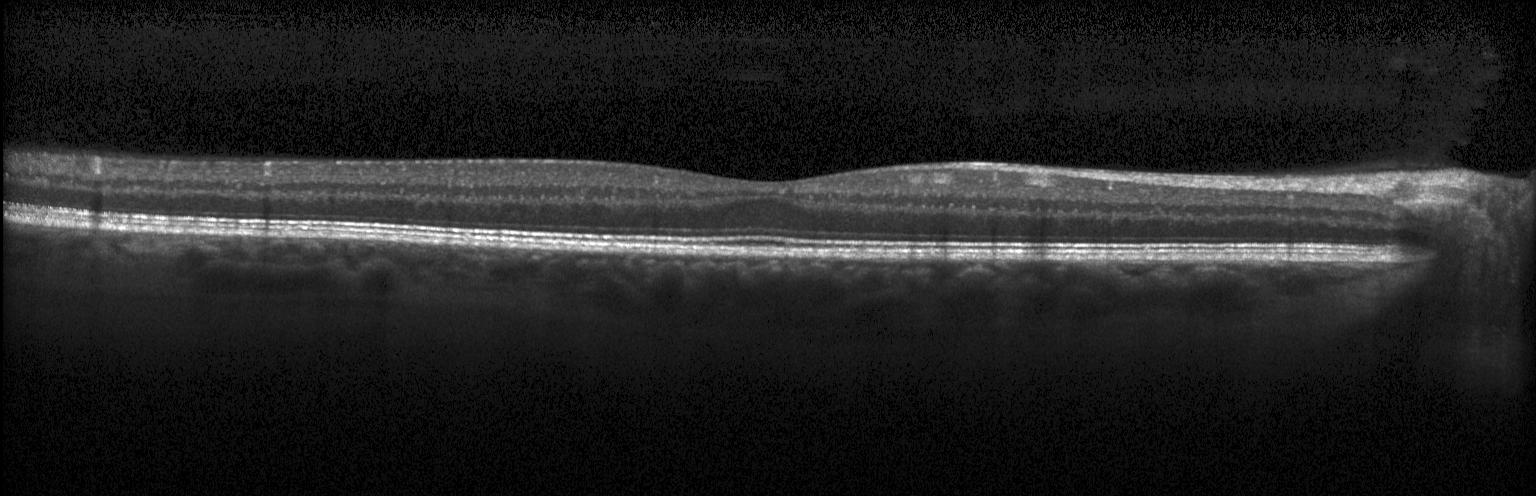 Optical coherence tomography B-scan.
Assessment: no CNV, DME, or drusen.